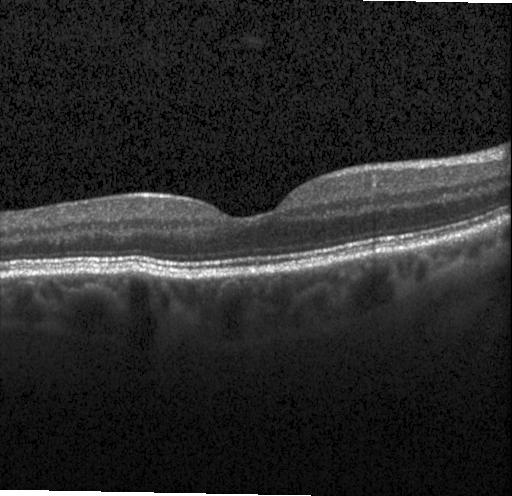

Retinal OCT B-scan; Heidelberg Spectralis OCT system; macular scan; spectral-domain OCT — Finding: no evidence of choroidal neovascularization, diabetic macular edema, or drusen.